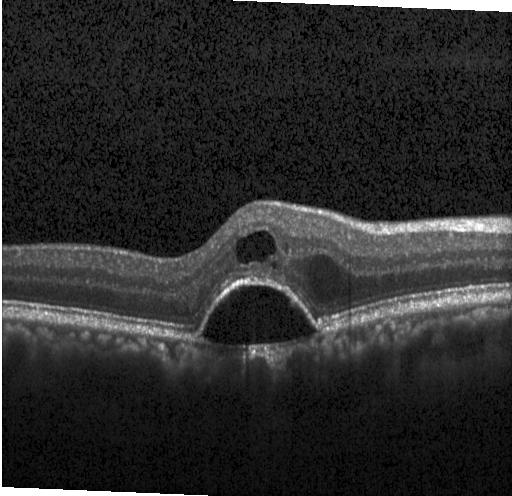 OCT line scan, acquired on a Heidelberg Spectralis.
A choroidal neovascular membrane.